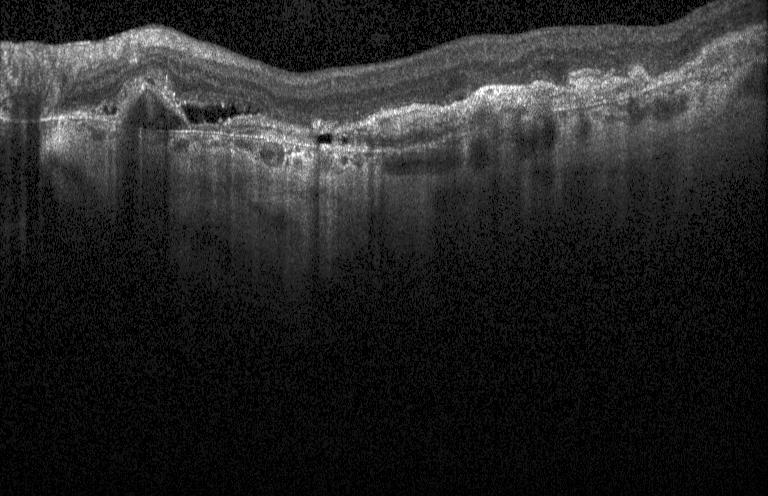 Impression: a choroidal neovascular membrane.